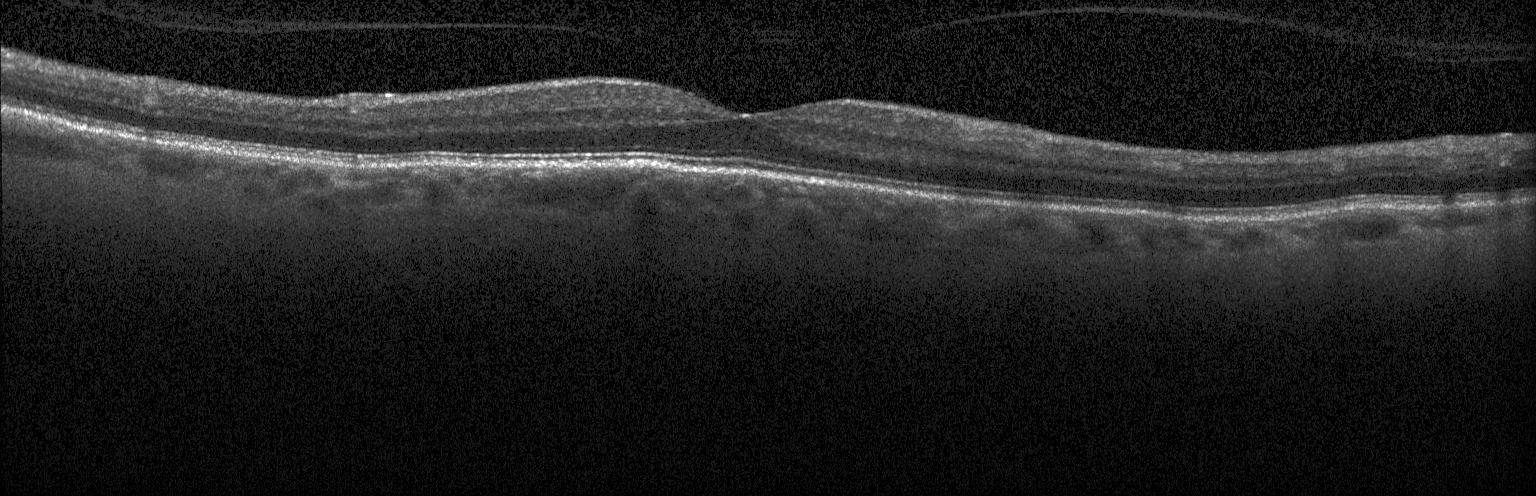 Through the macula, optical coherence tomography scan.
Assessment: no evidence of choroidal neovascularization, diabetic macular edema, or drusen.